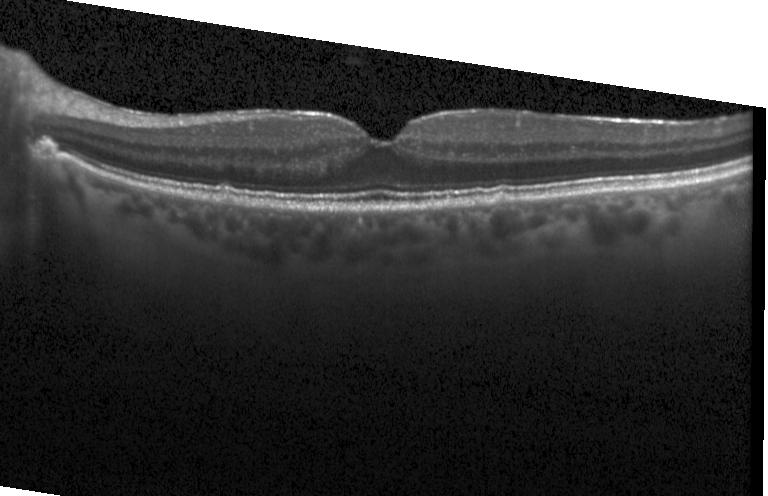
Diagnosis: no CNV, no DME, and no drusen.